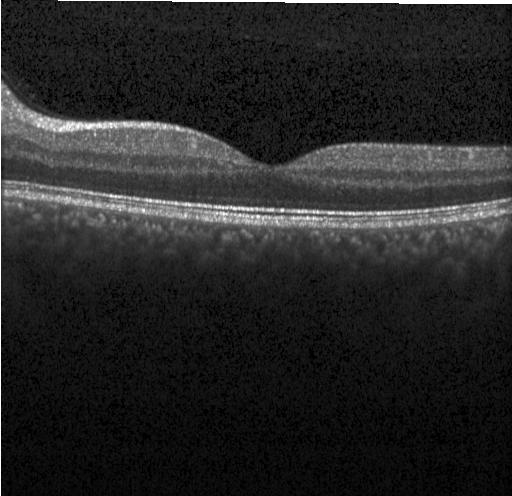

Dx: neither CNV, DME, nor drusen.